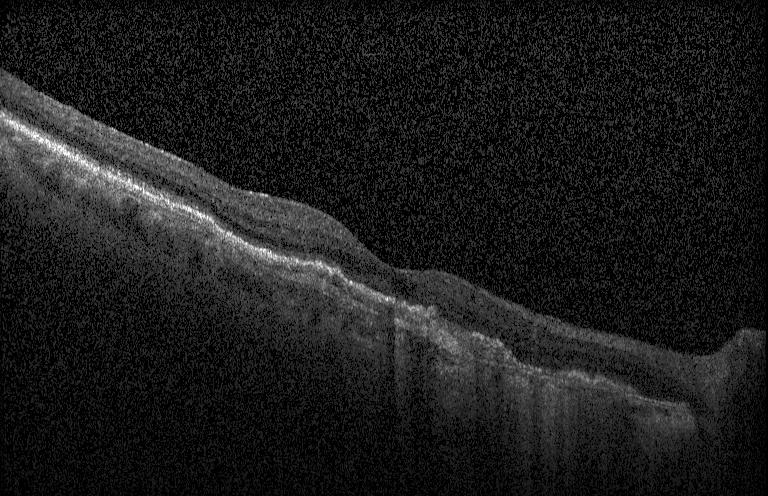

Through the macula, Heidelberg Spectralis OCT system, retinal OCT cross-section, SD-OCT. This B-scan demonstrates CNV.